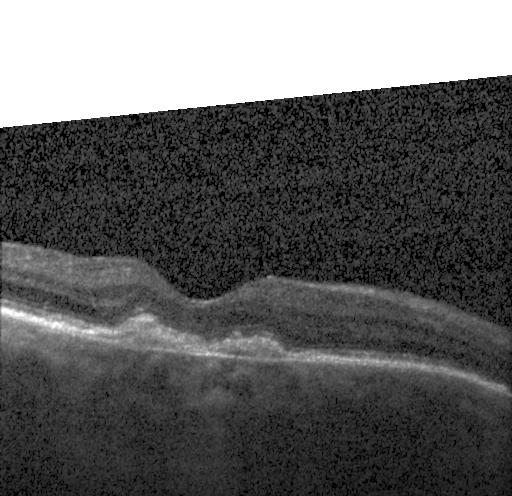
OCT finding: a choroidal neovascular membrane.